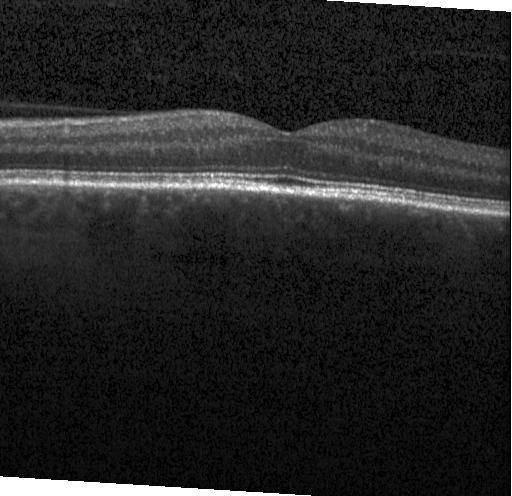

Macular scan. Acquired on a Heidelberg Spectralis. Spectral-domain optical coherence tomography. Optical coherence tomography B-scan. OCT finding: no choroidal neovascularization, diabetic macular edema, or drusen.